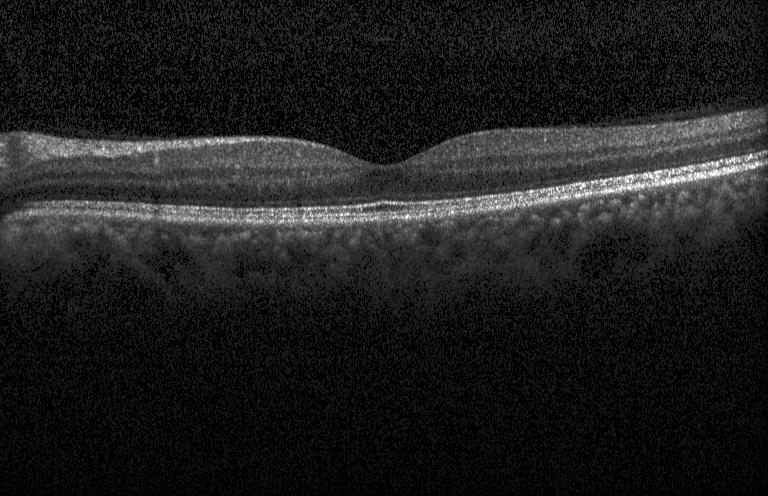

Heidelberg Spectralis OCT system; optical coherence tomography scan; spectral-domain optical coherence tomography; horizontal scan through the fovea — This B-scan demonstrates no choroidal neovascularization, diabetic macular edema, or drusen.